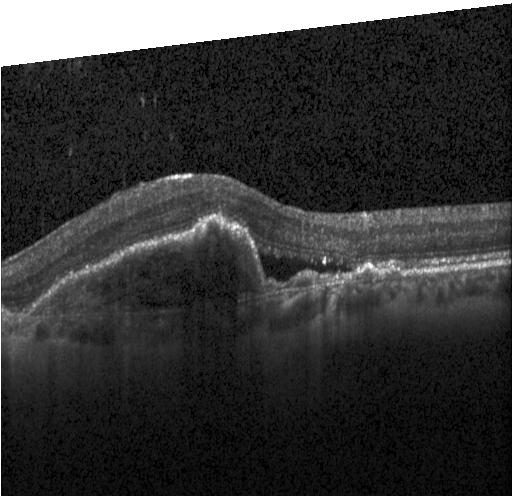

Spectral-domain optical coherence tomography, horizontal scan through the fovea, optical coherence tomography B-scan. This B-scan demonstrates a choroidal neovascular membrane.